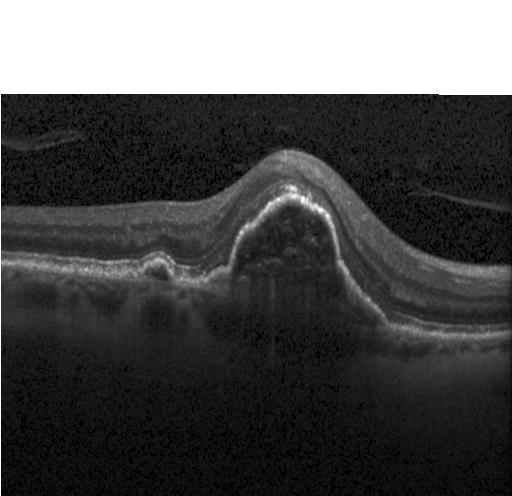

Spectral-domain OCT B-scan: a choroidal neovascular membrane.